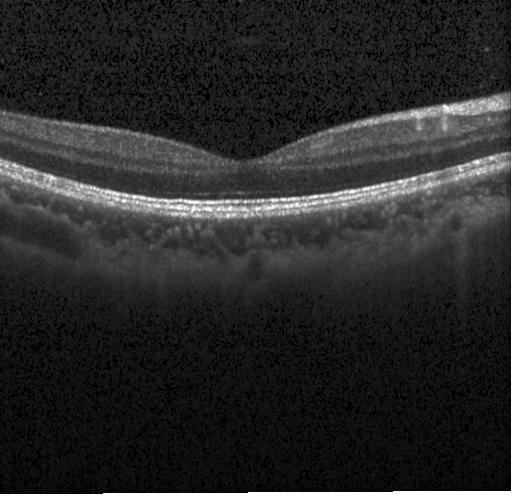

Spectral-domain OCT, optical coherence tomography B-scan
Diagnosis: no evidence of choroidal neovascularization, diabetic macular edema, or drusen.